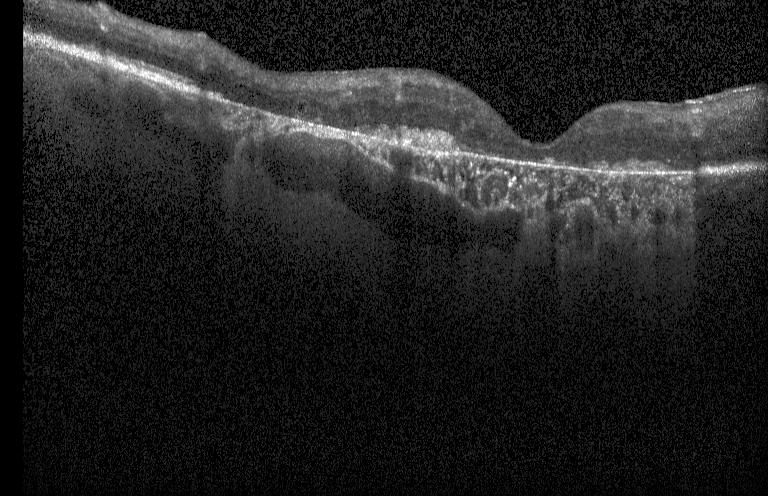
Heidelberg Spectralis; SD-OCT; OCT line scan; through the macula. Impression: CNV.